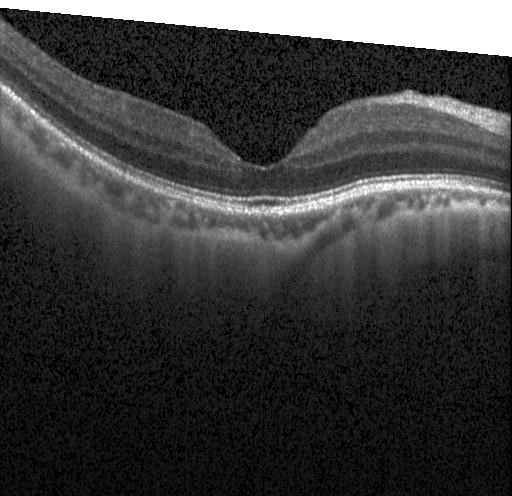 Spectral-domain OCT B-scan: no CNV, DME, or drusen.